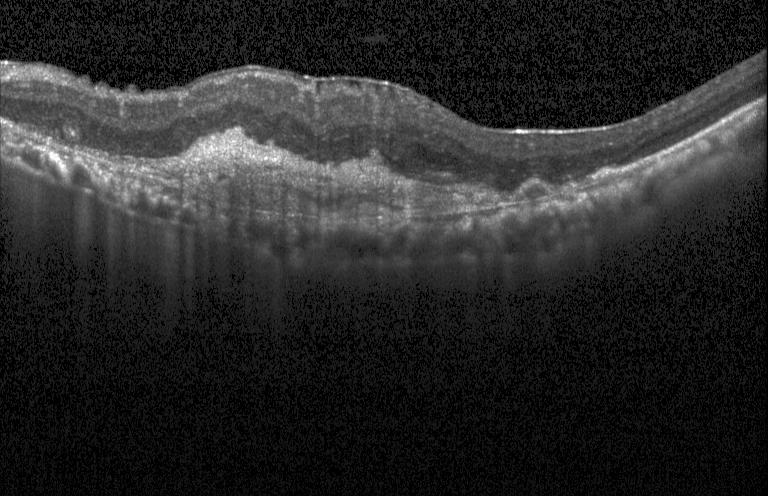 Spectral-domain OCT B-scan: CNV.